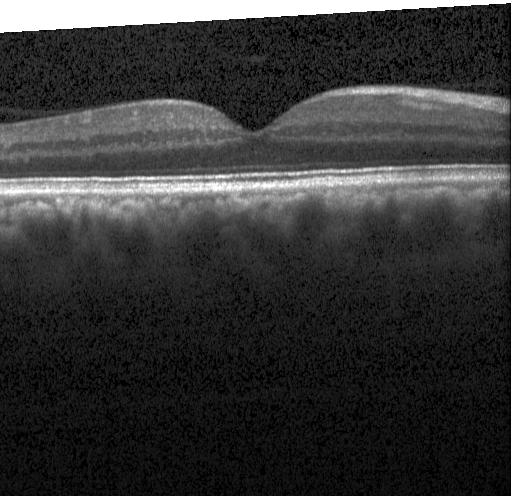

Macular OCT demonstrating no CNV, DME, or drusen.